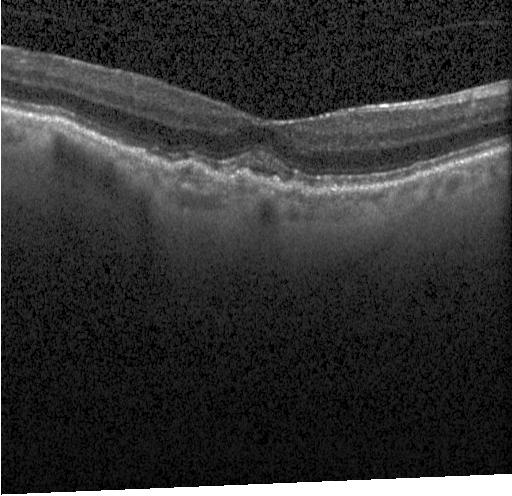 Acquired on a Heidelberg Spectralis; OCT line scan; spectral-domain OCT. Diagnosis: CNV.